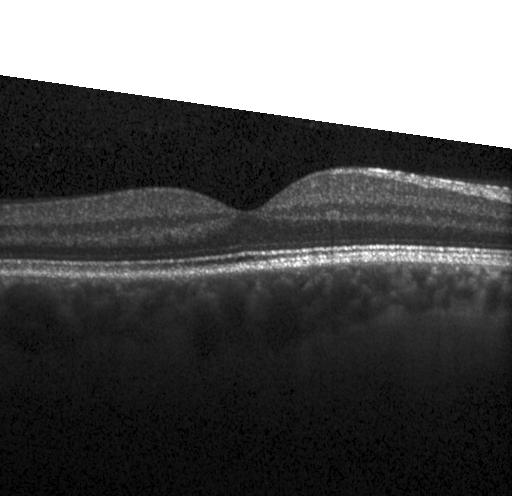

SD-OCT, OCT line scan, fovea-centered
Dx: no choroidal neovascularization, no diabetic macular edema, and no drusen.